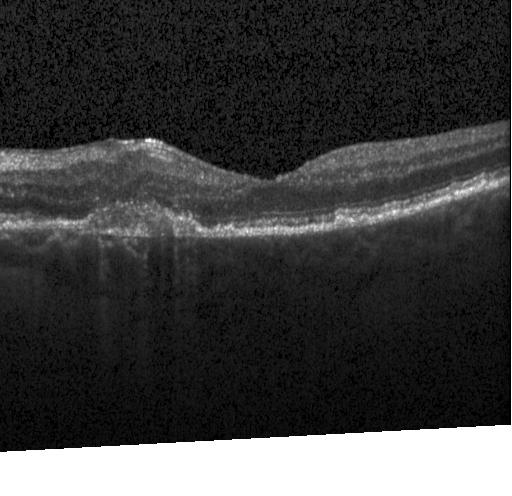
Retinal OCT B-scan · fovea-centered
Choroidal neovascularization.